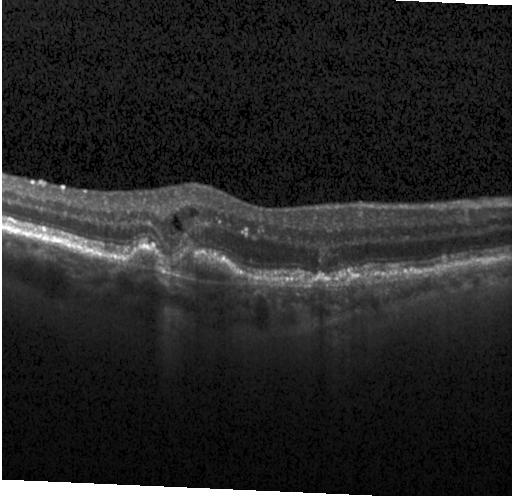
OCT finding: choroidal neovascularization (CNV).